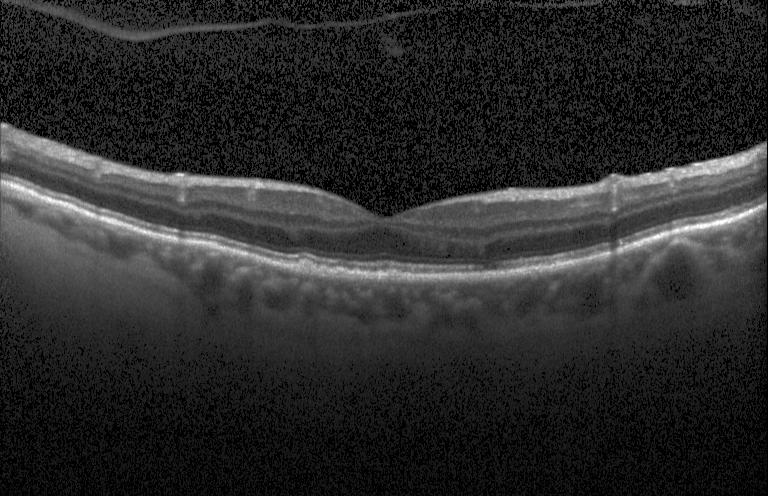
OCT line scan — Diagnosis: drusen.